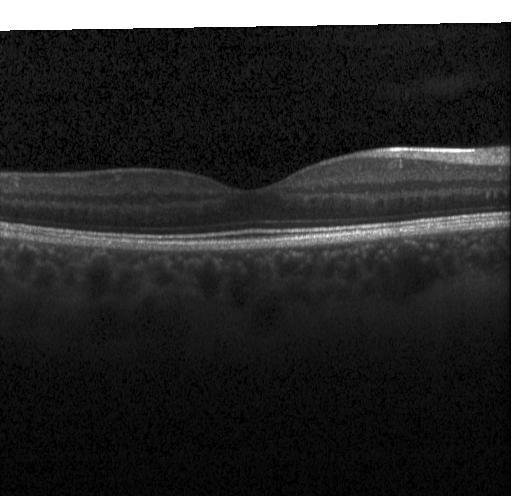

Acquired on a Heidelberg Spectralis, centered on the fovea, OCT B-scan, spectral-domain OCT — Finding: no choroidal neovascularization, no diabetic macular edema, and no drusen.